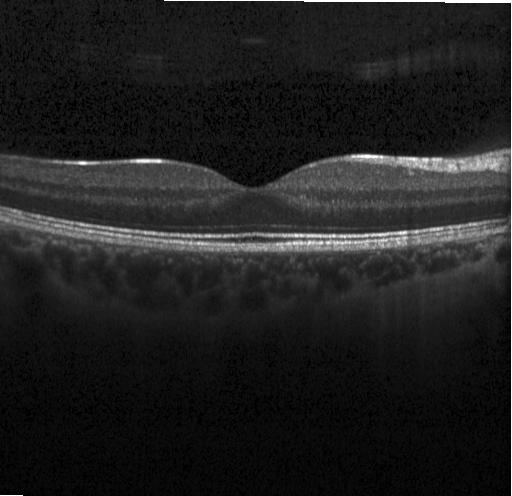 OCT scan showing neither CNV, DME, nor drusen.